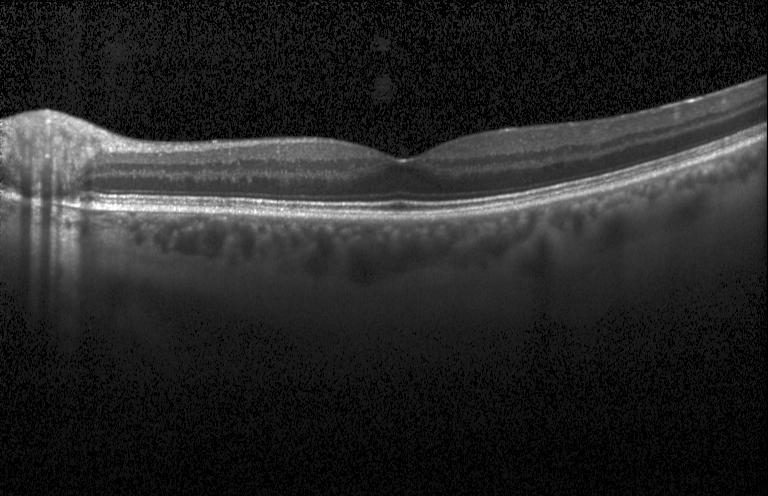 Retinal OCT B-scan · acquired on a Heidelberg Spectralis · SD-OCT · macular scan. Finding: no evidence of choroidal neovascularization, diabetic macular edema, or drusen.